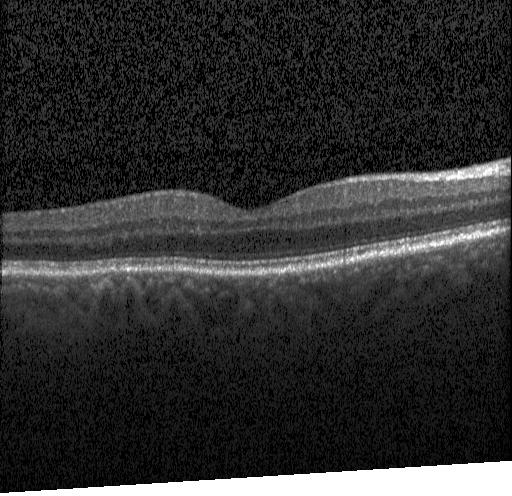
Centered on the fovea · OCT line scan · instrument: Heidelberg Spectralis · spectral-domain OCT.
Impression: no evidence of choroidal neovascularization, diabetic macular edema, or drusen.